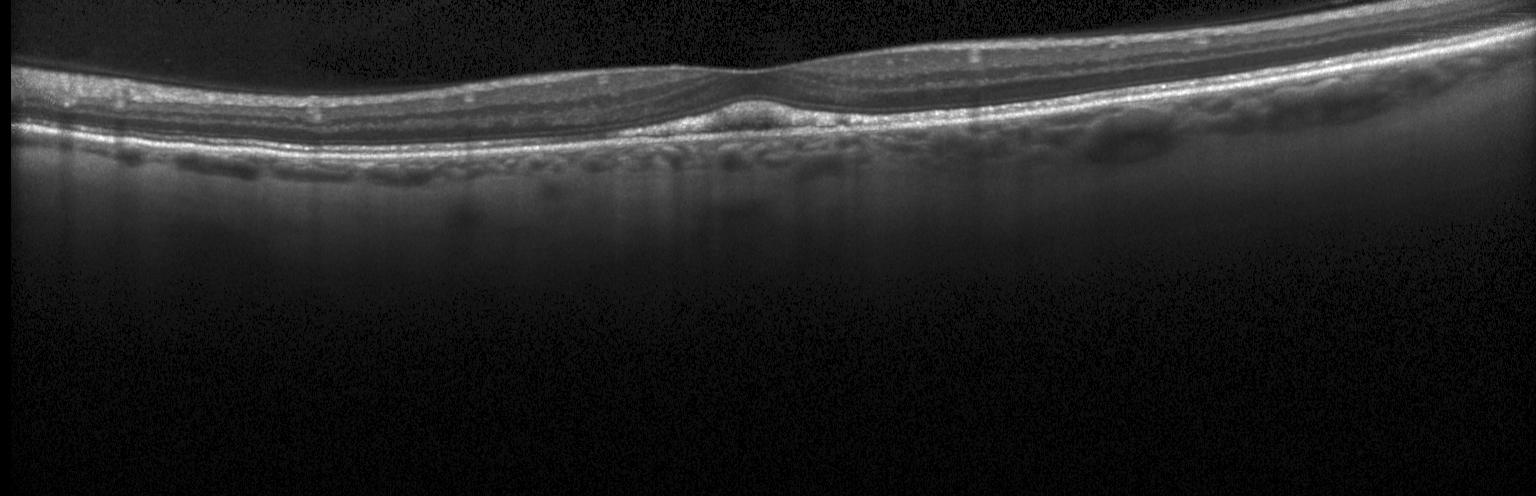

Spectral-domain OCT B-scan: a choroidal neovascular membrane.